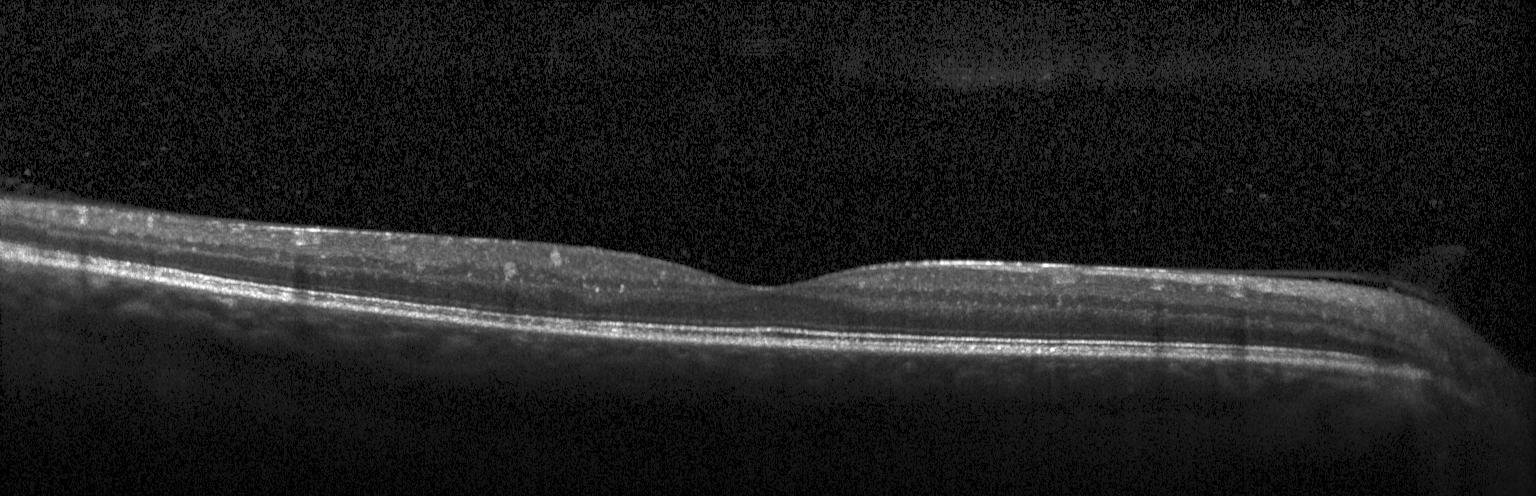
Retinal OCT cross-section. The scan shows neither choroidal neovascularization, diabetic macular edema, nor drusen.